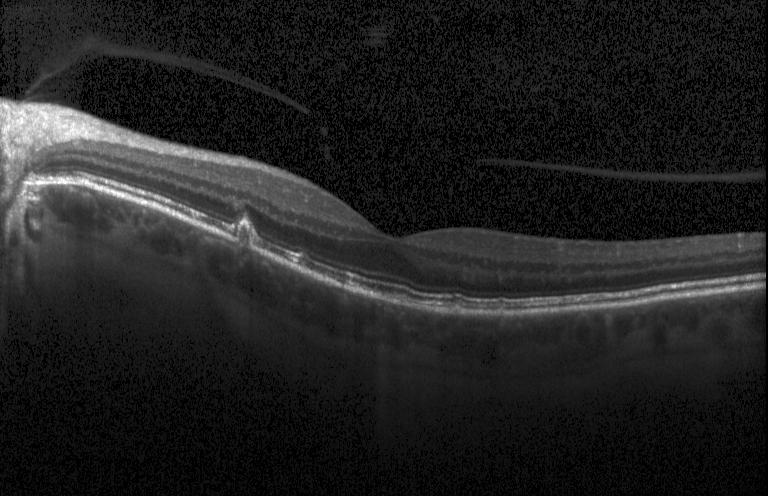 Optical coherence tomography scan · SD-OCT
Finding: drusen.